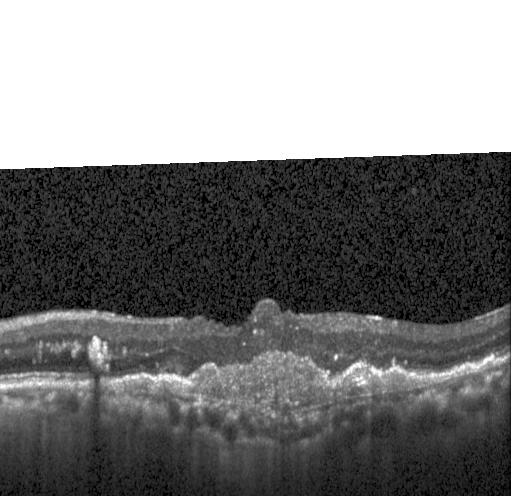 Spectral-domain optical coherence tomography. Acquired on a Heidelberg Spectralis. Retinal OCT B-scan — Dx: choroidal neovascularization.